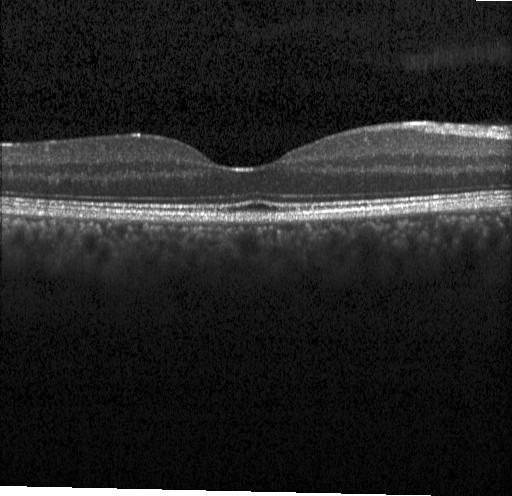 OCT B-scan showing neither choroidal neovascularization, diabetic macular edema, nor drusen.